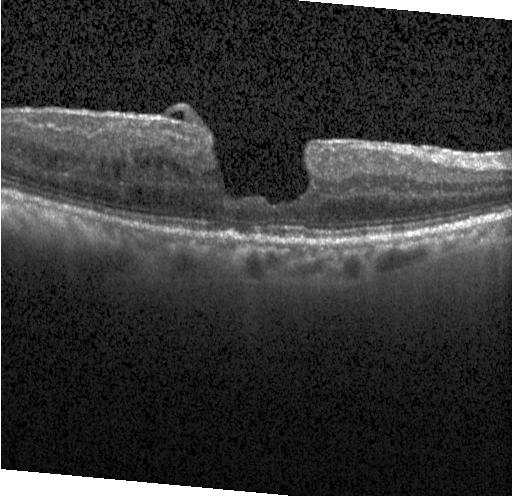
Dx: diabetic macular edema.